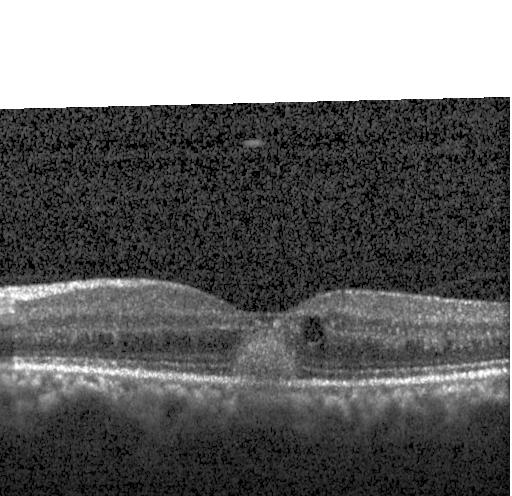

Diagnosis: CNV.